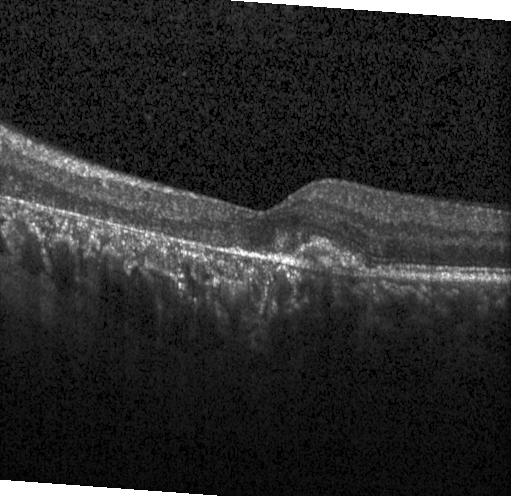
OCT finding: a choroidal neovascular membrane.